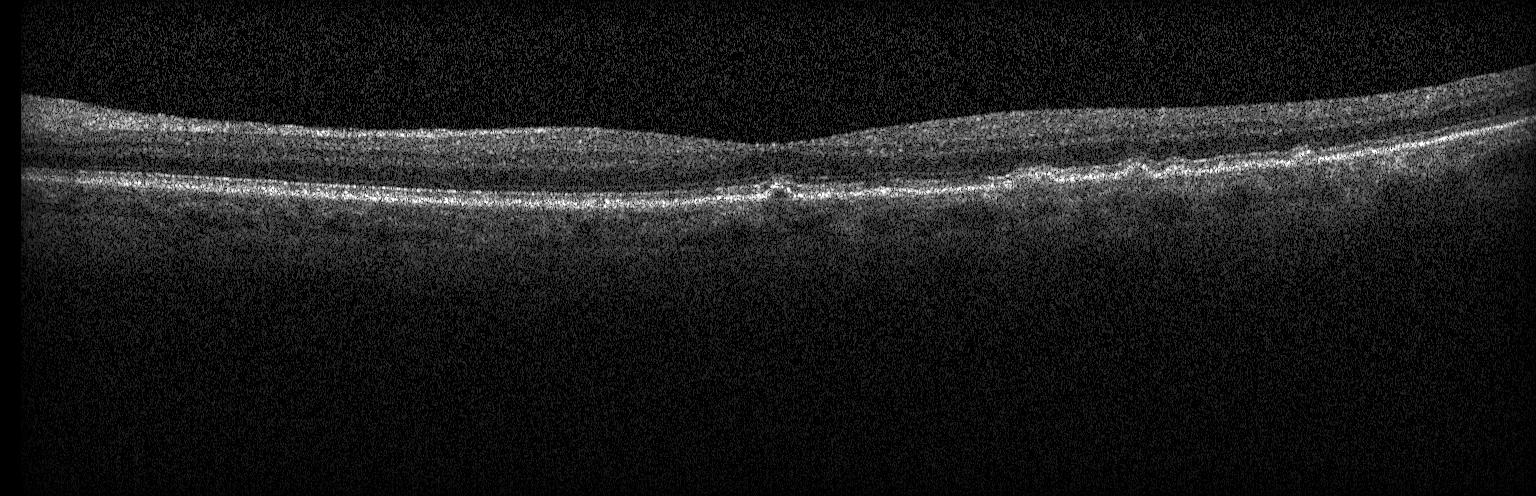

Drusen.